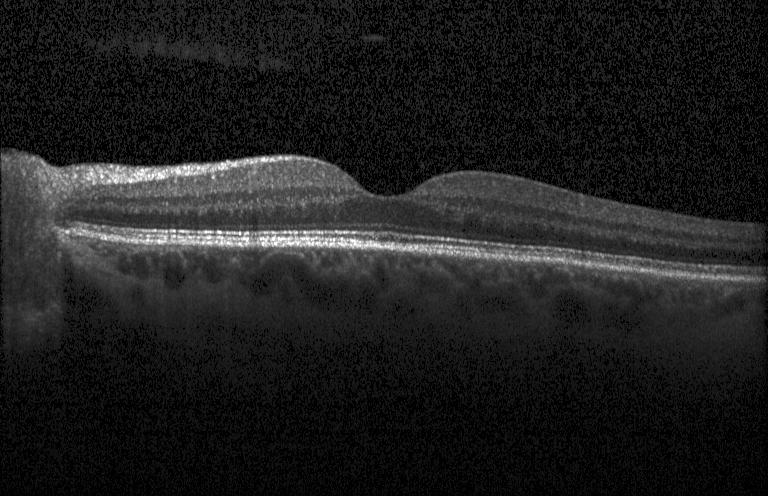

Heidelberg Spectralis. SD-OCT. OCT line scan. Horizontal scan through the fovea
Dx: no CNV, DME, or drusen.